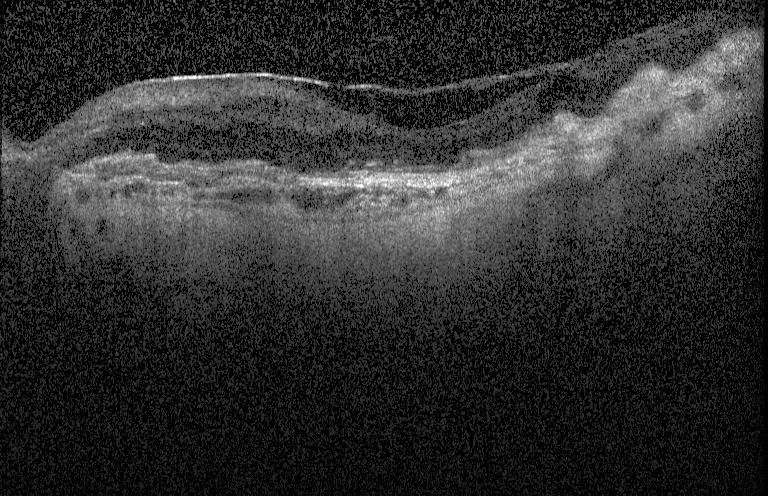

Retinal OCT cross-section showing a choroidal neovascular membrane.